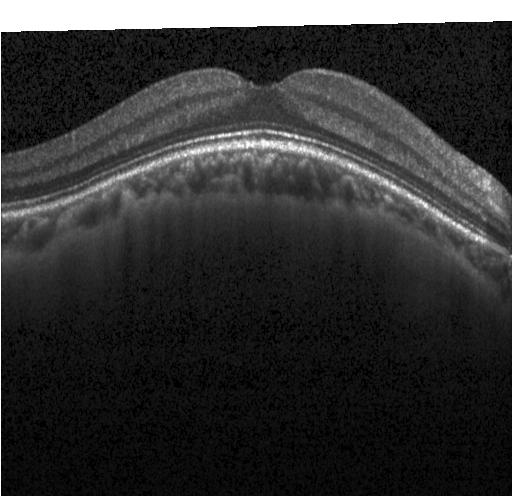 Diagnosis: no choroidal neovascularization, no diabetic macular edema, and no drusen.